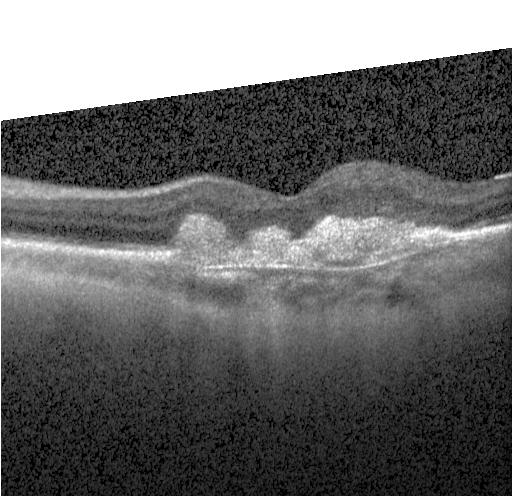 Spectral-domain OCT; retinal OCT cross-section; centered on the fovea; Heidelberg Spectralis OCT system.
A choroidal neovascular membrane.